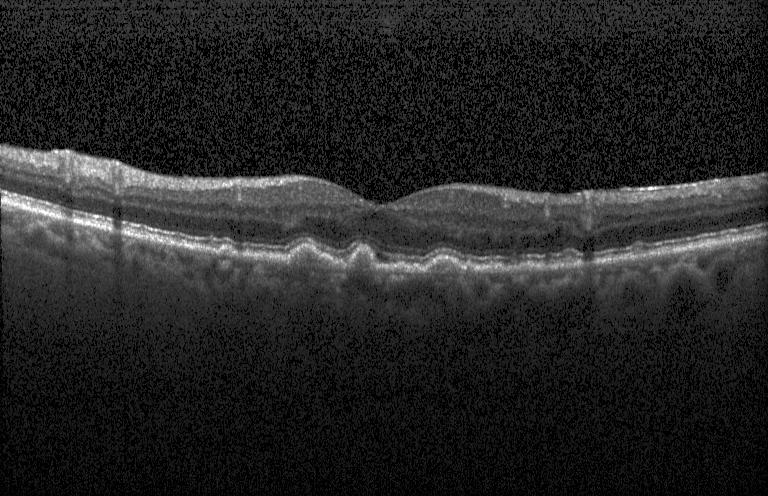

Diagnosis: drusen.